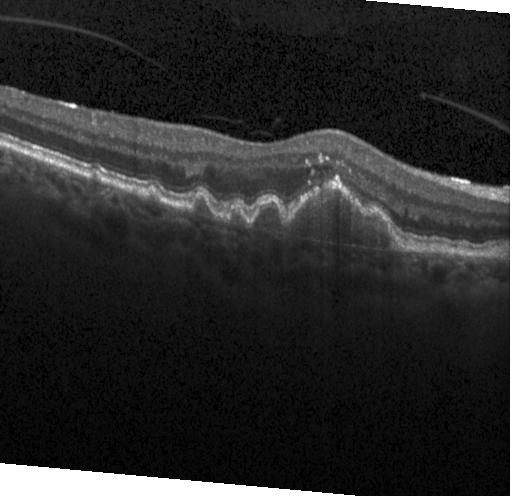

Macular OCT: choroidal neovascularization.